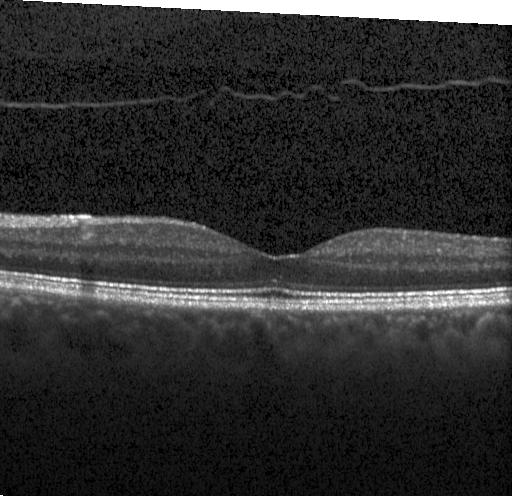 Impression: no CNV, no DME, and no drusen.